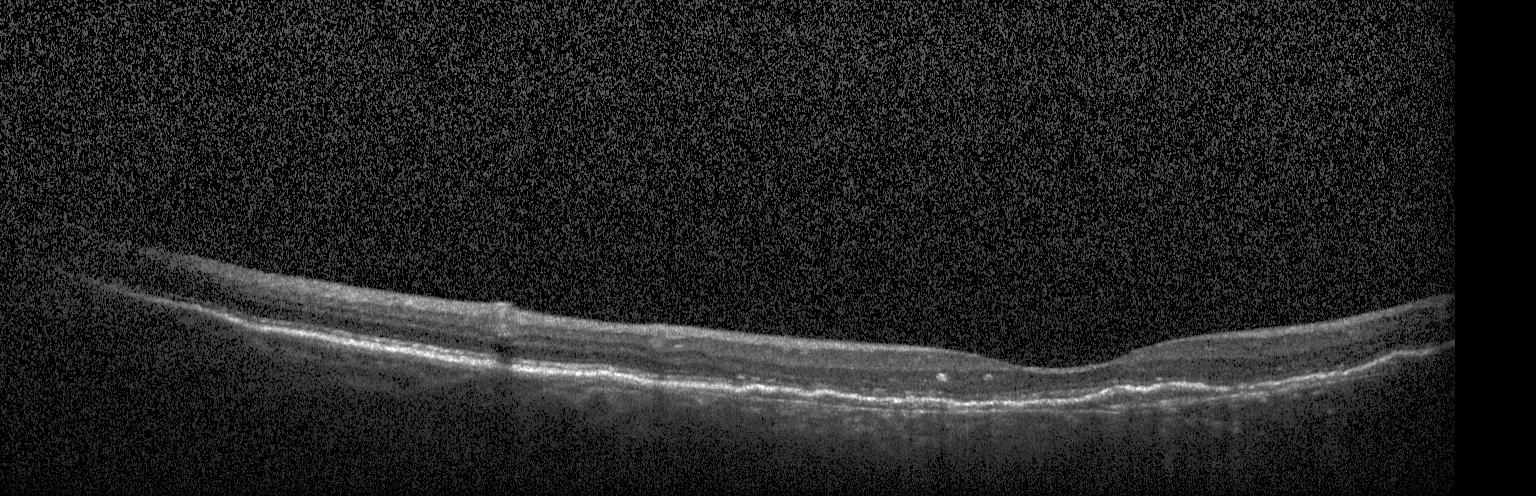
Fovea-centered · optical coherence tomography scan · spectral-domain optical coherence tomography.
Assessment: a choroidal neovascular membrane.